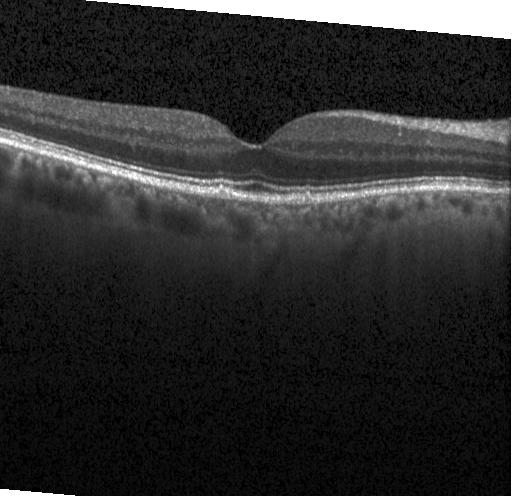 OCT B-scan. Spectral-domain optical coherence tomography — Diagnosis: drusen.